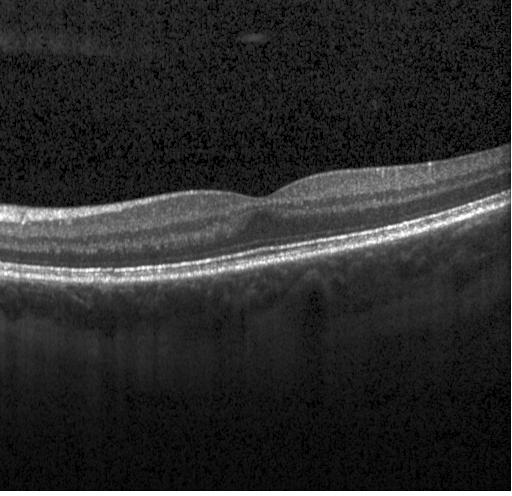 OCT B-scan
No evidence of choroidal neovascularization, diabetic macular edema, or drusen.